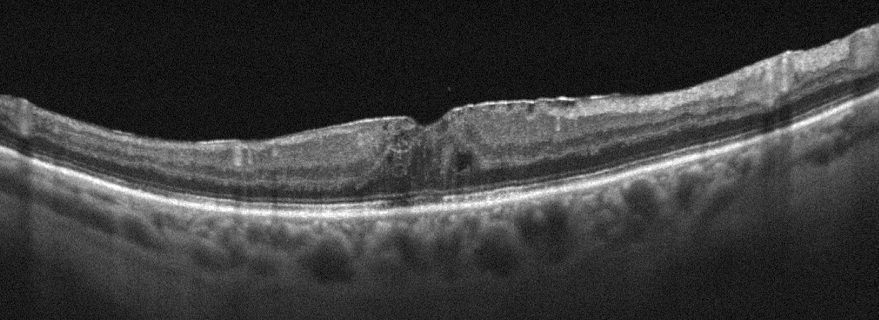
Retinal OCT cross-section showing epiretinal membrane (ERM).